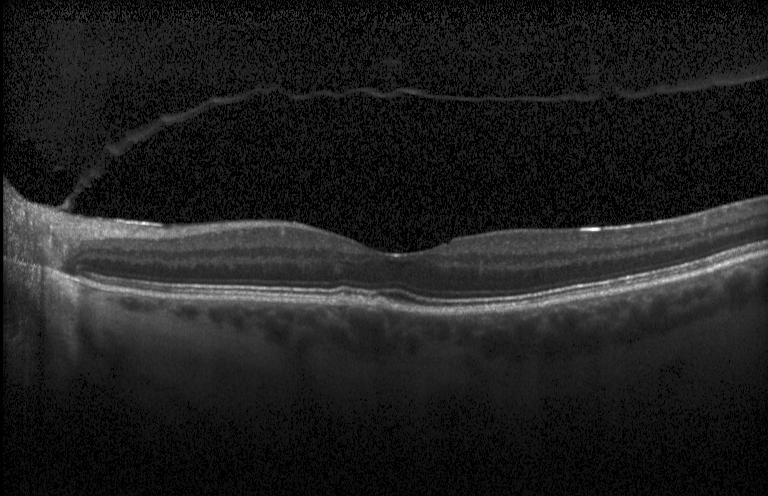
Spectral-domain optical coherence tomography; retinal OCT B-scan; centered on the fovea. This B-scan demonstrates multiple drusen.